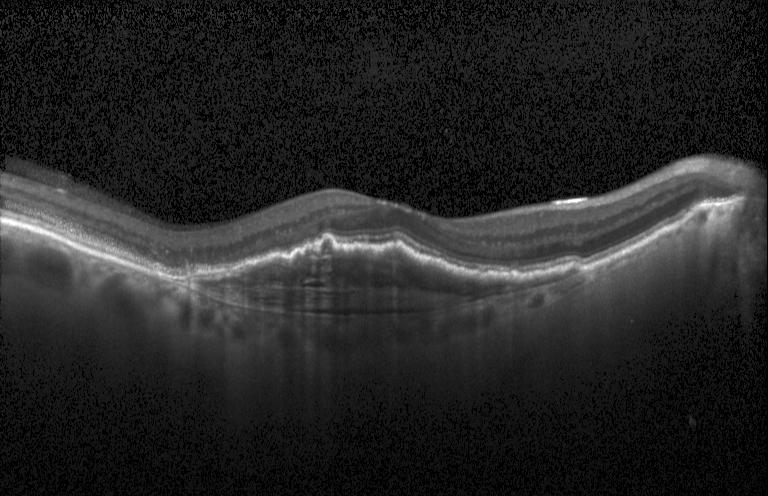
Impression: choroidal neovascularization.